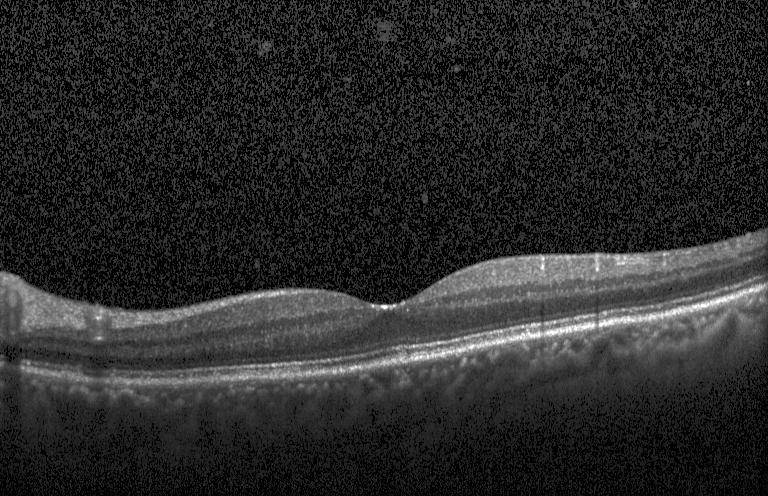
SD-OCT, OCT line scan.
Neither CNV, DME, nor drusen.